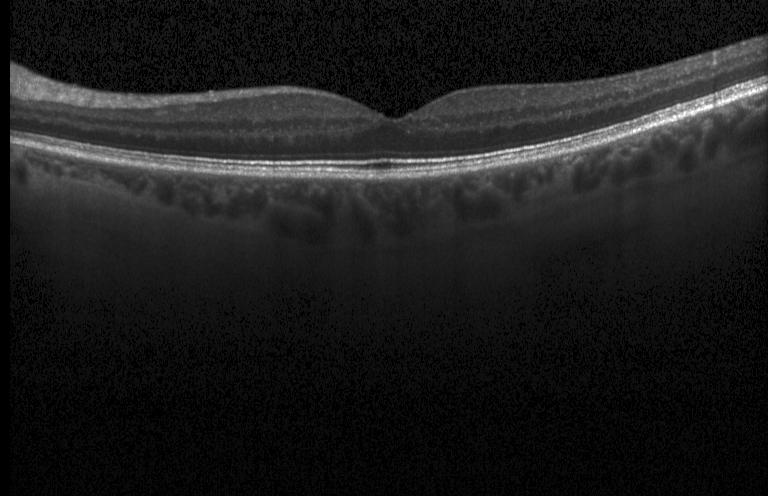
Spectral-domain OCT B-scan: neither choroidal neovascularization, diabetic macular edema, nor drusen.